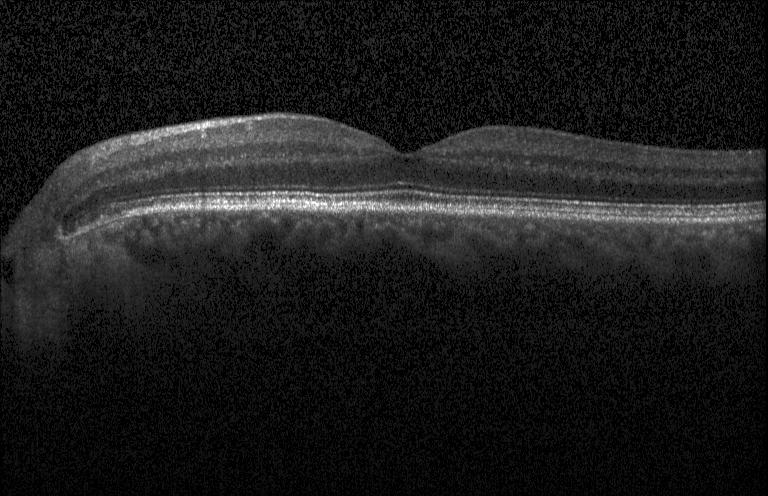 Optical coherence tomography B-scan. Diagnosis: no choroidal neovascularization, diabetic macular edema, or drusen.